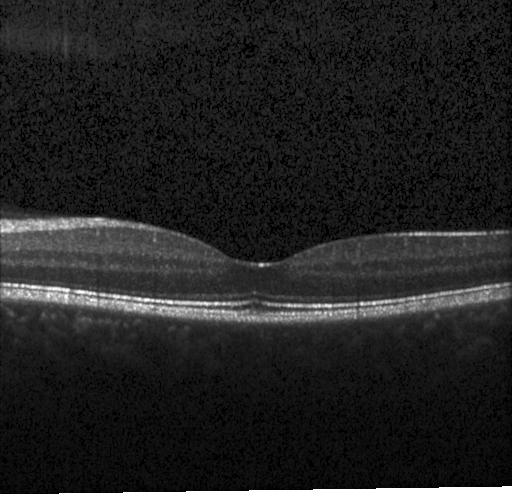 The scan shows no CNV, no DME, and no drusen.